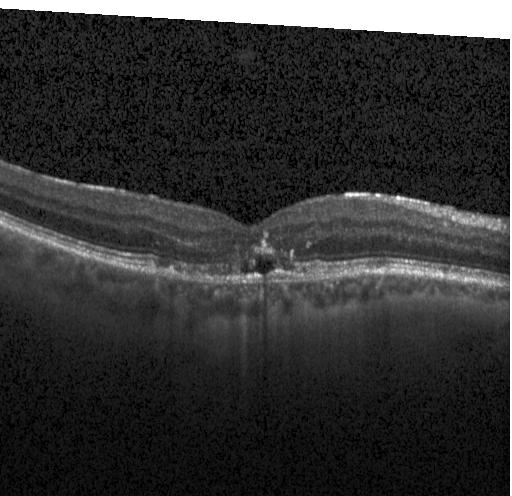 Fovea-centered · SD-OCT · optical coherence tomography B-scan
This B-scan demonstrates CNV.